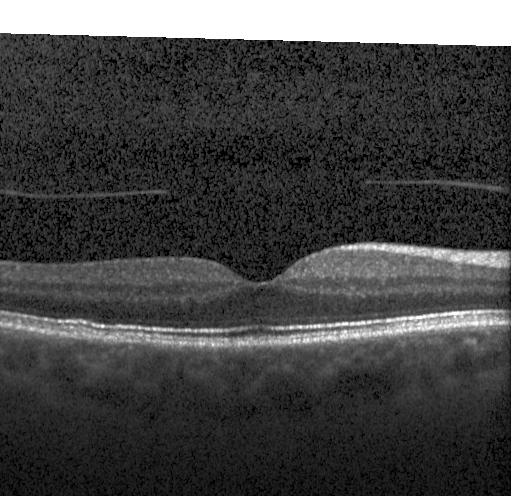 OCT B-scan showing neither CNV, DME, nor drusen.